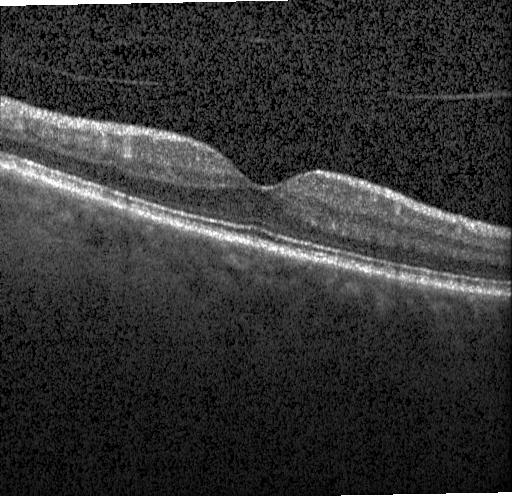 Diagnosis: no CNV, DME, or drusen.